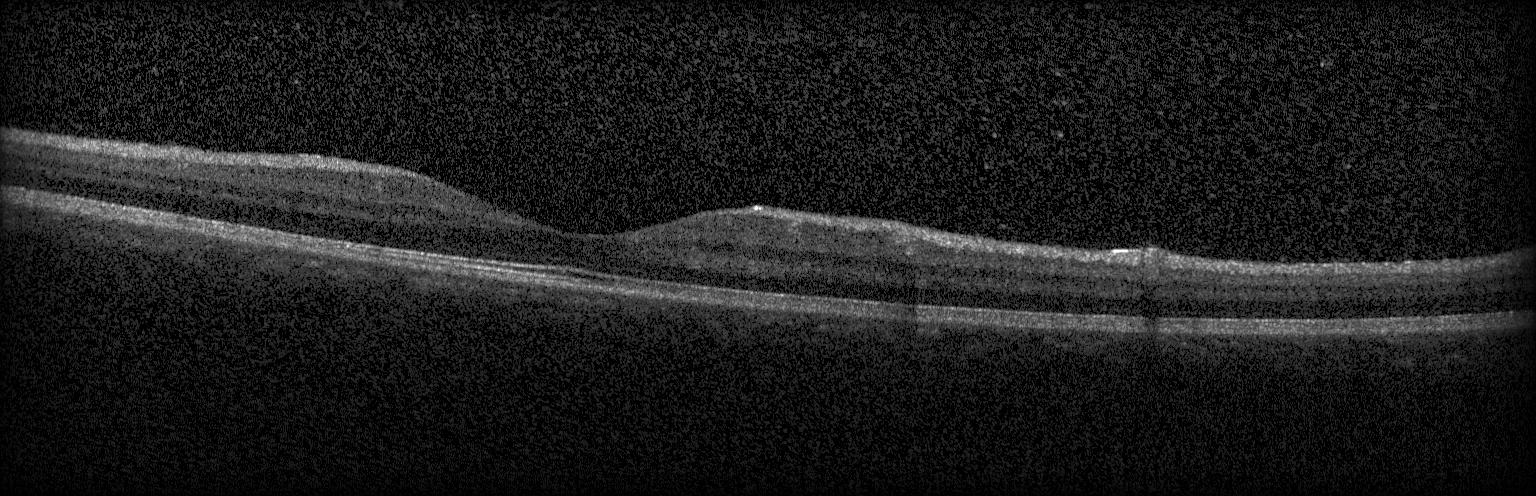 Finding: no choroidal neovascularization, diabetic macular edema, or drusen.